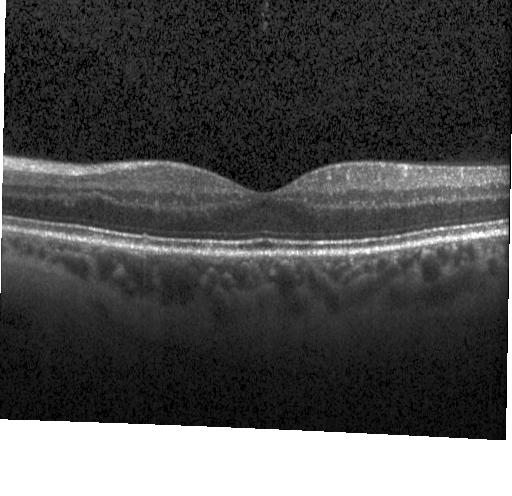 OCT B-scan · Heidelberg Spectralis OCT system · spectral-domain optical coherence tomography · macular scan
Diagnosis: no CNV, DME, or drusen.